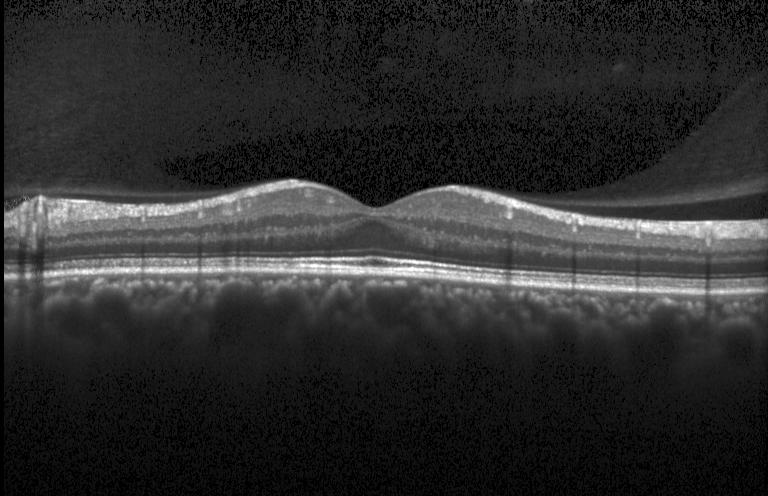

Optical coherence tomography B-scan · spectral-domain optical coherence tomography · centered on the fovea
Macular OCT: no choroidal neovascularization, no diabetic macular edema, and no drusen.